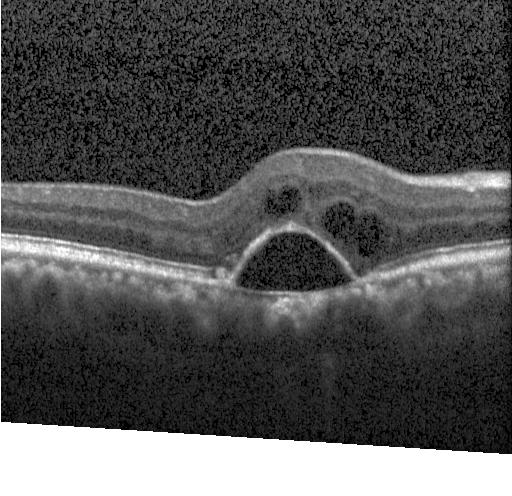

CNV.